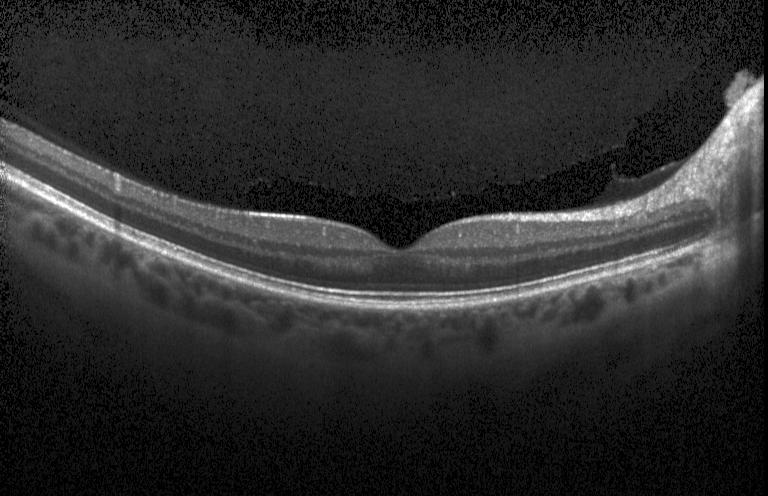

OCT B-scan; instrument: Heidelberg Spectralis; SD-OCT; centered on the fovea.
This B-scan demonstrates no choroidal neovascularization, no diabetic macular edema, and no drusen.